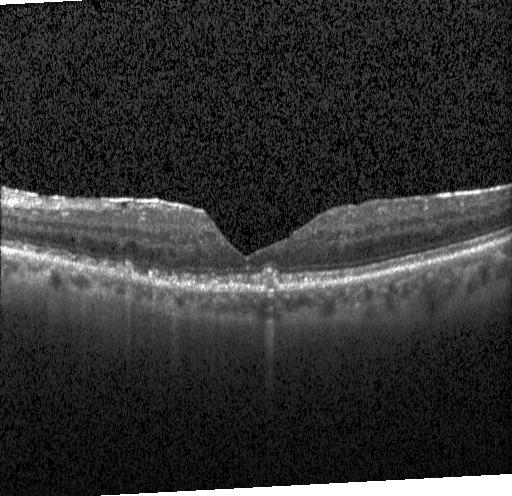 Retinal OCT cross-section showing multiple drusen.